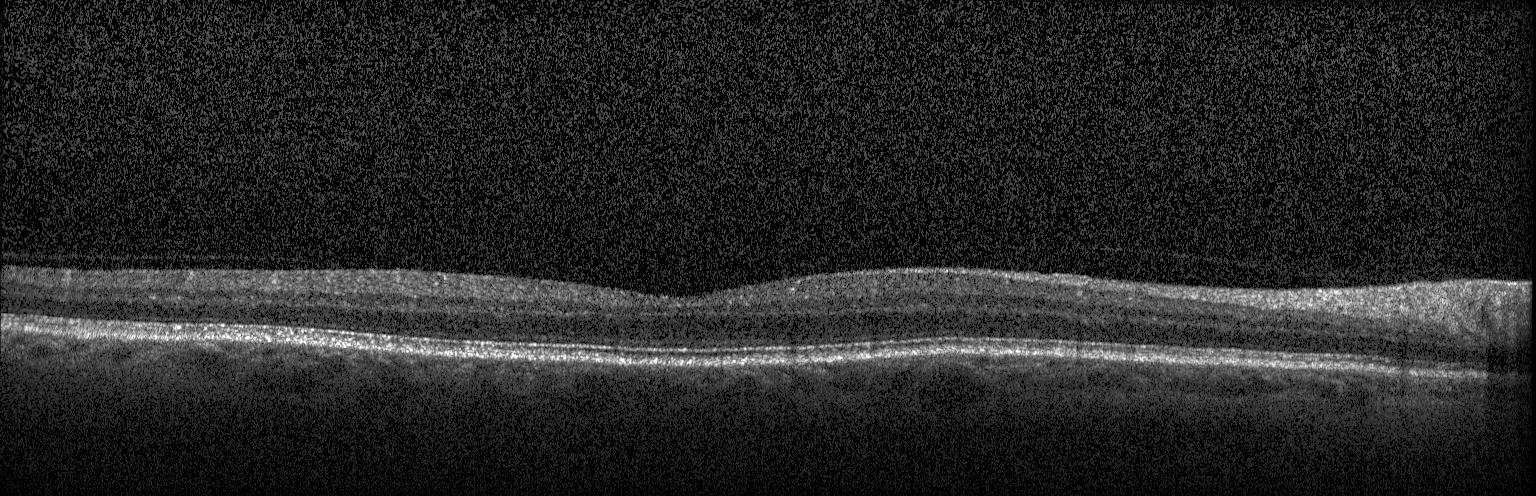

Heidelberg Spectralis, fovea-centered, optical coherence tomography scan, SD-OCT.
This B-scan demonstrates no choroidal neovascularization, no diabetic macular edema, and no drusen.